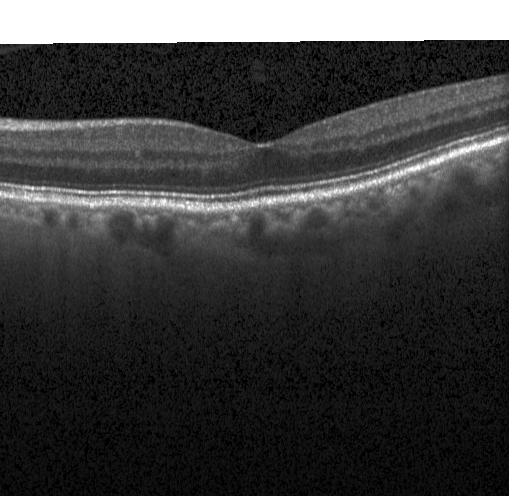
Macular scan; optical coherence tomography B-scan; acquired on a Heidelberg Spectralis.
Finding: neither choroidal neovascularization, diabetic macular edema, nor drusen.